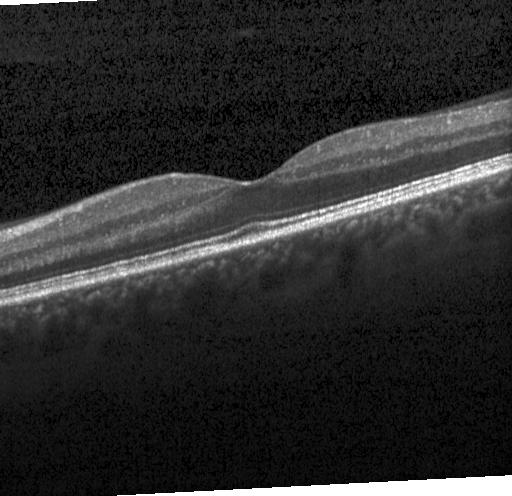

Optical coherence tomography B-scan · centered on the fovea · spectral-domain optical coherence tomography · Heidelberg Spectralis — Dx: no CNV, no DME, and no drusen.